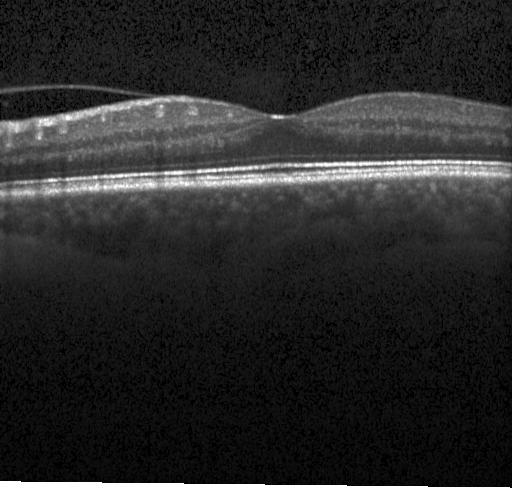
Retinal OCT cross-section — Assessment: no evidence of choroidal neovascularization, diabetic macular edema, or drusen.